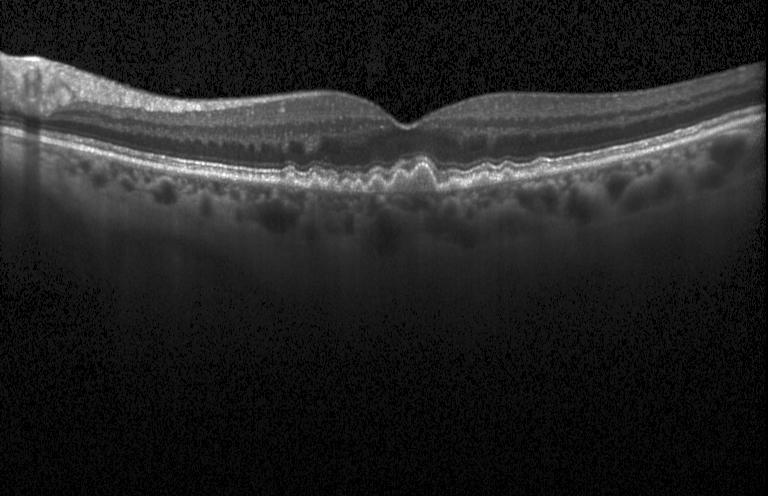 Horizontal scan through the fovea · retinal OCT B-scan · Heidelberg Spectralis — Assessment: drusen.